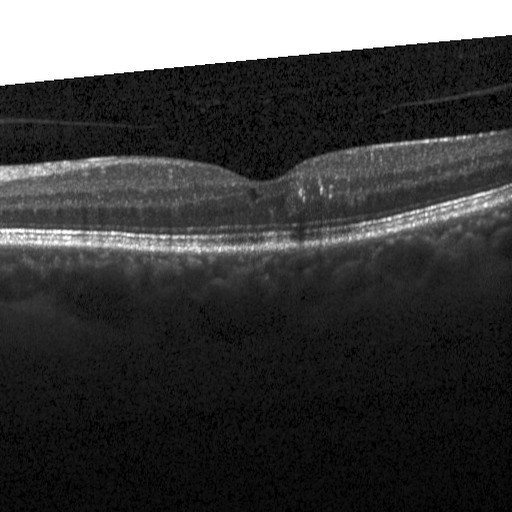

Finding: diabetic macular edema (DME).